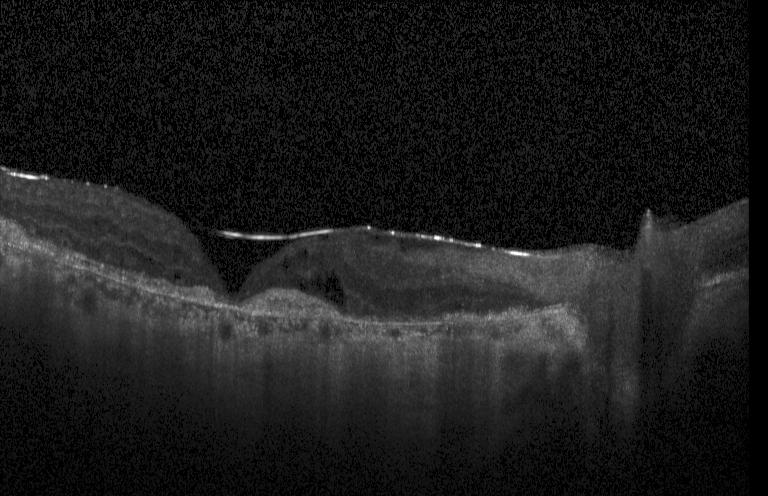 OCT B-scan; spectral-domain OCT; centered on the fovea.
Impression: CNV.